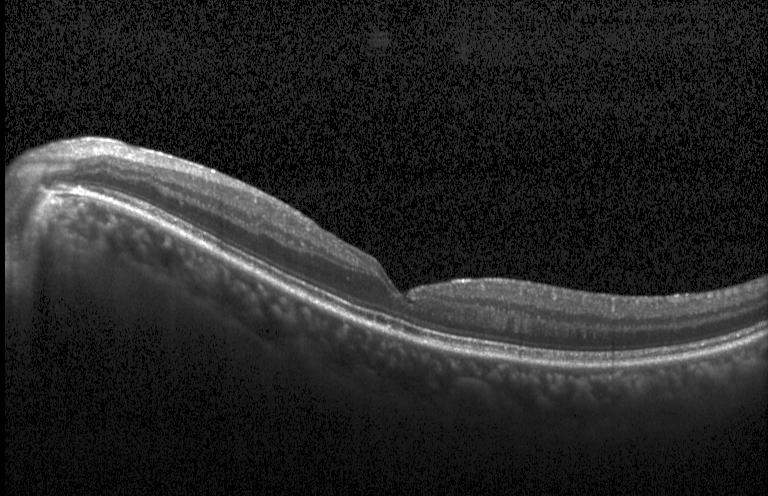

Spectral-domain OCT; optical coherence tomography B-scan; fovea-centered — Assessment: no evidence of choroidal neovascularization, diabetic macular edema, or drusen.